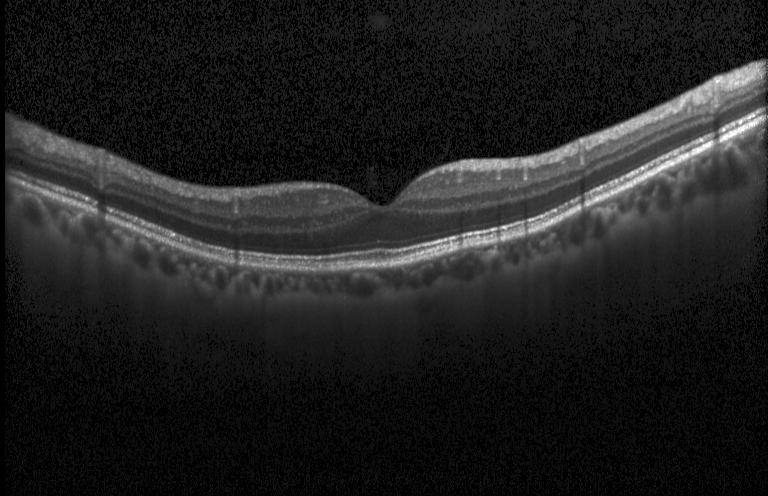 Impression: no evidence of choroidal neovascularization, diabetic macular edema, or drusen.